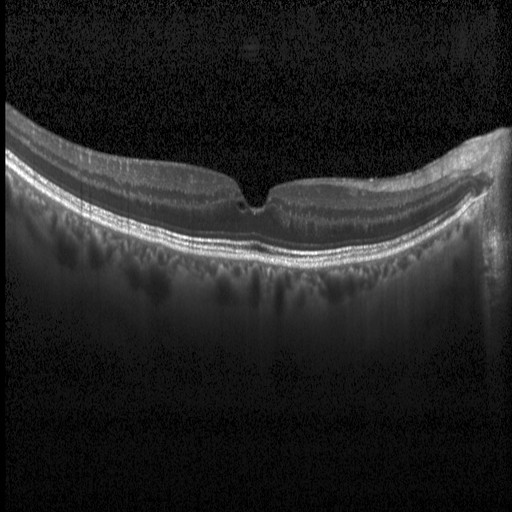 Macular OCT demonstrating diabetic macular edema (DME).